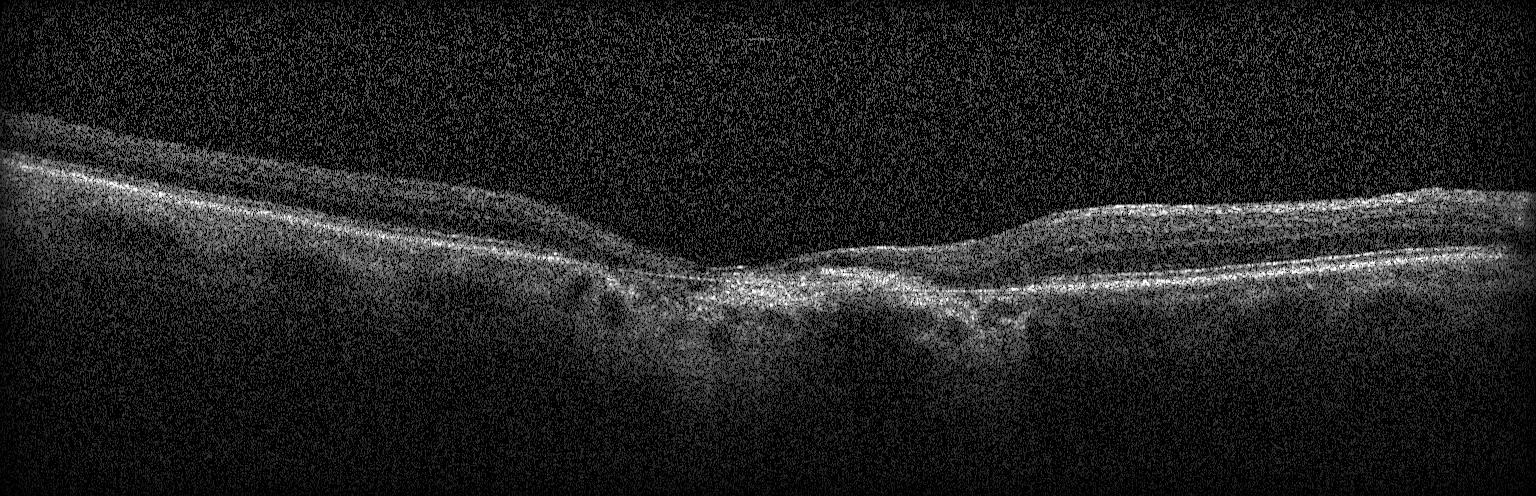
OCT line scan. Macular scan — This B-scan demonstrates a choroidal neovascular membrane.